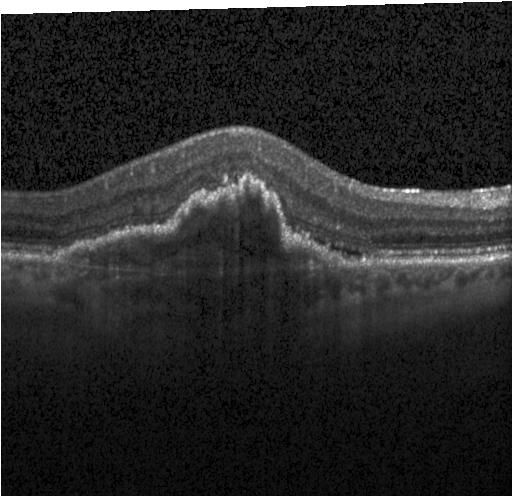
OCT B-scan. Acquired on a Heidelberg Spectralis
The scan shows a choroidal neovascular membrane.